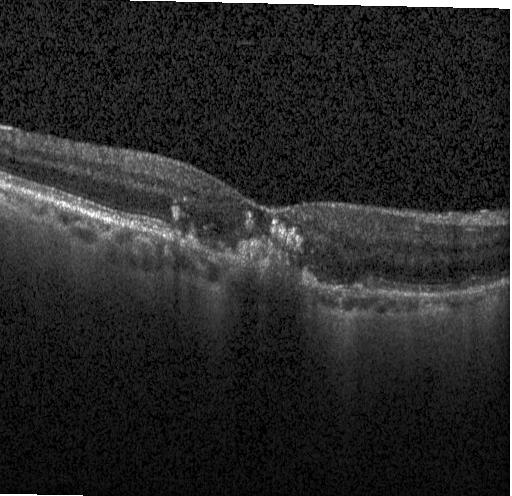

SD-OCT; Heidelberg Spectralis; centered on the fovea; optical coherence tomography scan — Macular OCT: a choroidal neovascular membrane.